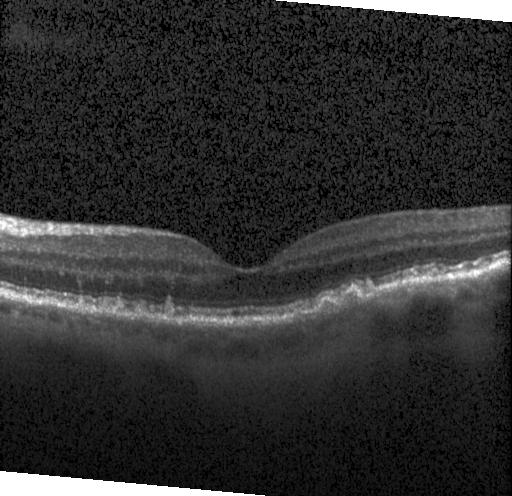

Optical coherence tomography scan · SD-OCT · instrument: Heidelberg Spectralis. This B-scan demonstrates sub-RPE drusenoid deposits.